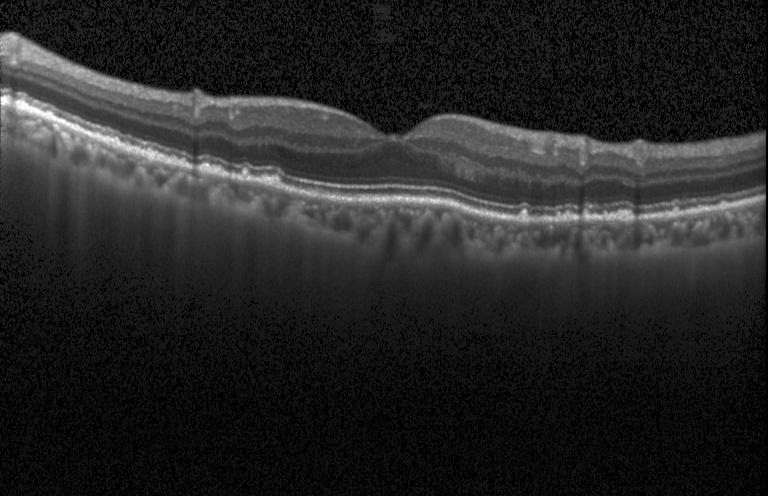 Macular OCT: multiple drusen.